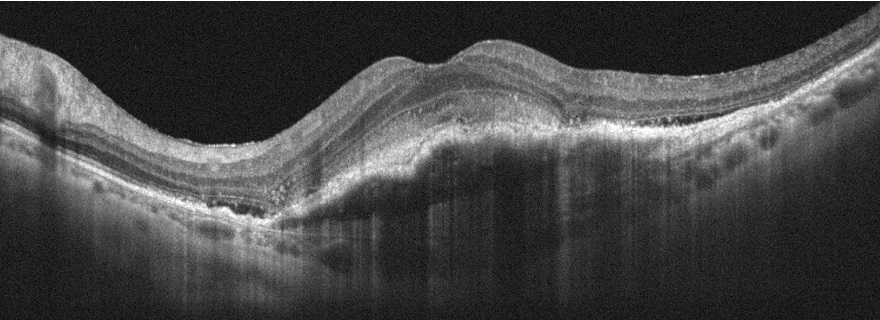

Diagnosis: AMD.